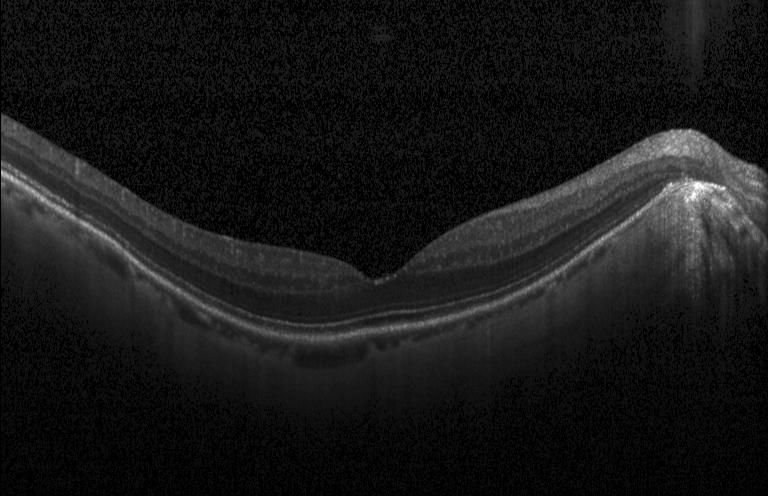
Optical coherence tomography scan. Heidelberg Spectralis OCT system — Diagnosis: no choroidal neovascularization, diabetic macular edema, or drusen.